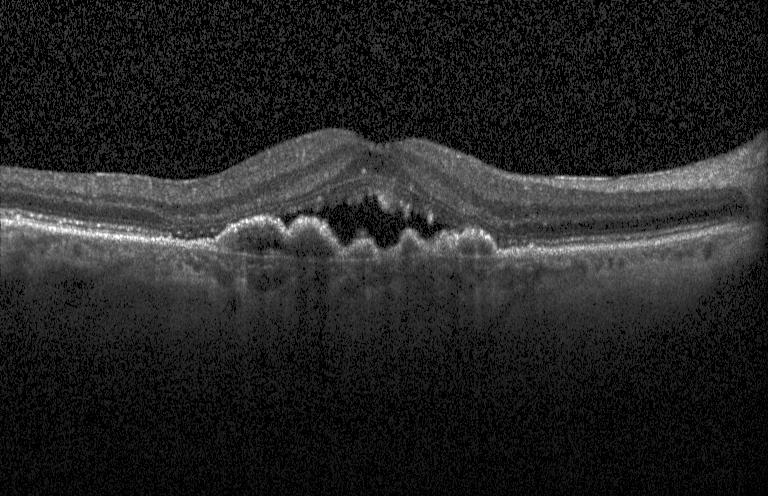 Impression: a choroidal neovascular membrane.